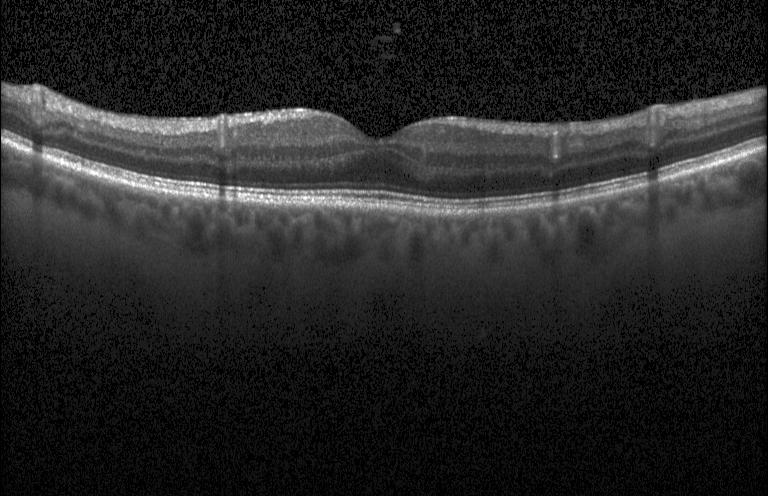
Spectral-domain OCT B-scan: no choroidal neovascularization, no diabetic macular edema, and no drusen.